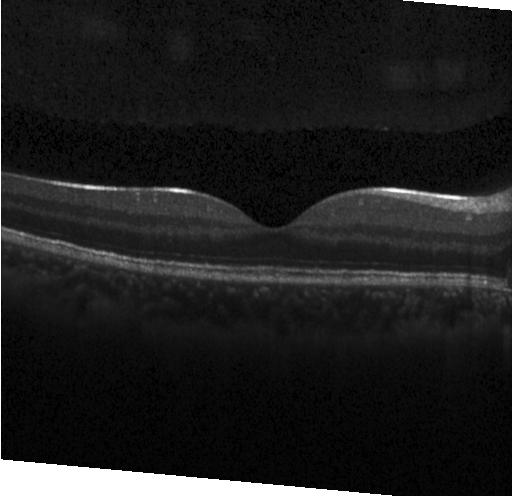
OCT B-scan showing no evidence of choroidal neovascularization, diabetic macular edema, or drusen.